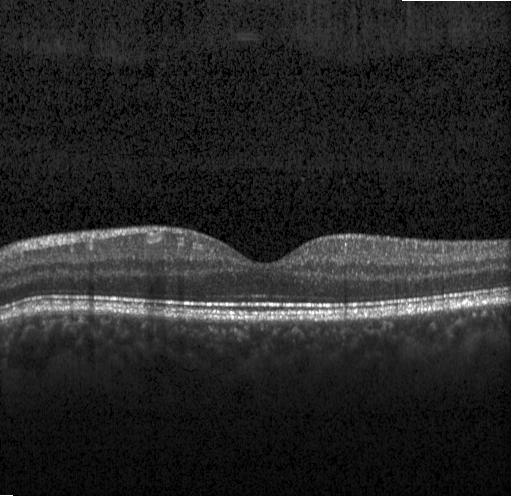 Heidelberg Spectralis OCT system · spectral-domain optical coherence tomography · OCT B-scan — OCT finding: no evidence of choroidal neovascularization, diabetic macular edema, or drusen.